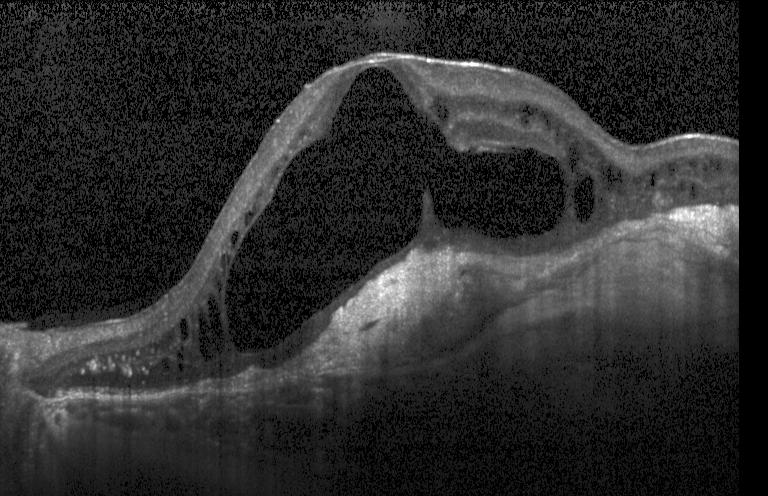 Retinal OCT B-scan
Finding: a choroidal neovascular membrane.